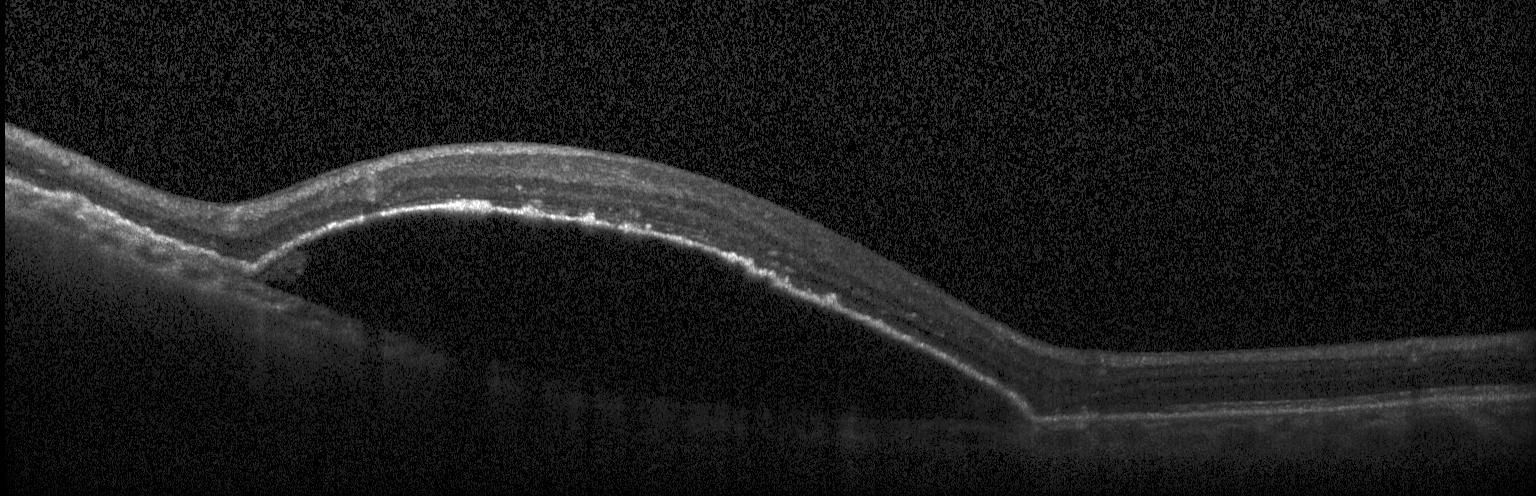 OCT B-scan showing a choroidal neovascular membrane.